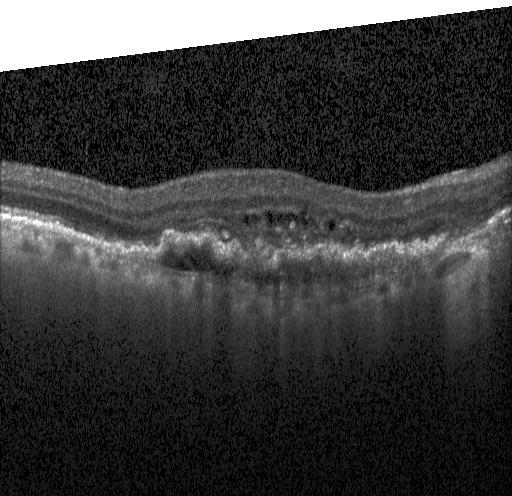
Dx: a choroidal neovascular membrane.